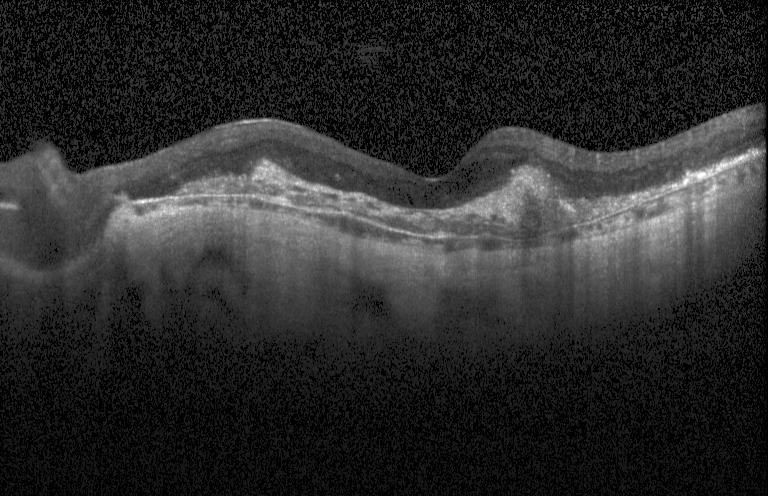
Optical coherence tomography B-scan — Finding: a choroidal neovascular membrane.